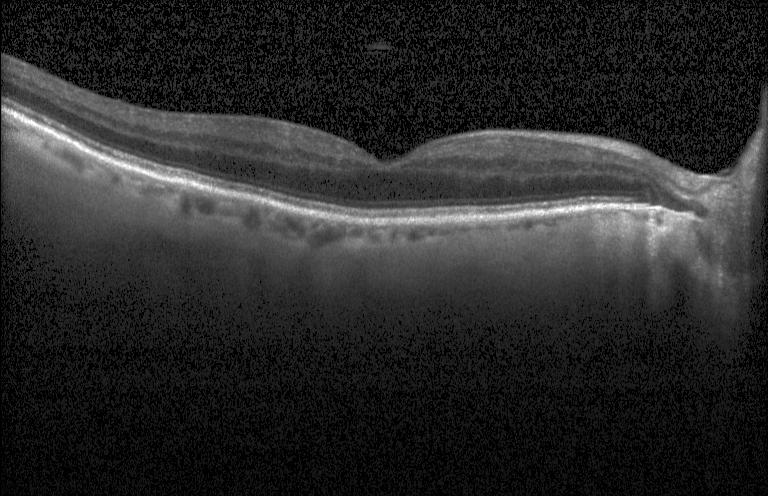 OCT line scan. Impression: no choroidal neovascularization, diabetic macular edema, or drusen.